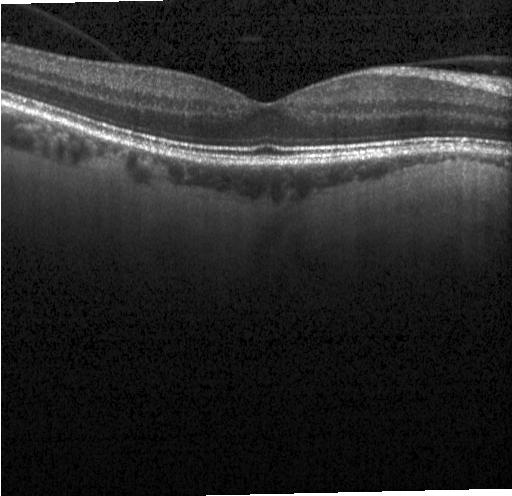 Retinal OCT cross-section — Diagnosis: neither CNV, DME, nor drusen.